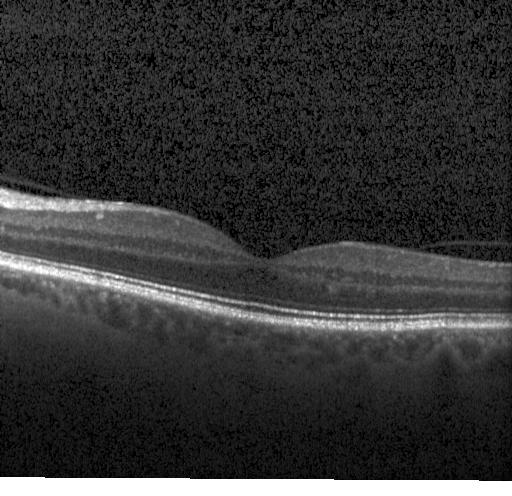 Macular OCT: no choroidal neovascularization, diabetic macular edema, or drusen.